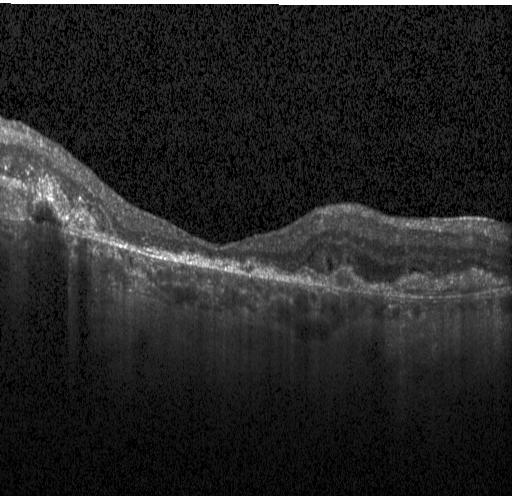

OCT line scan · instrument: Heidelberg Spectralis — Impression: choroidal neovascularization.